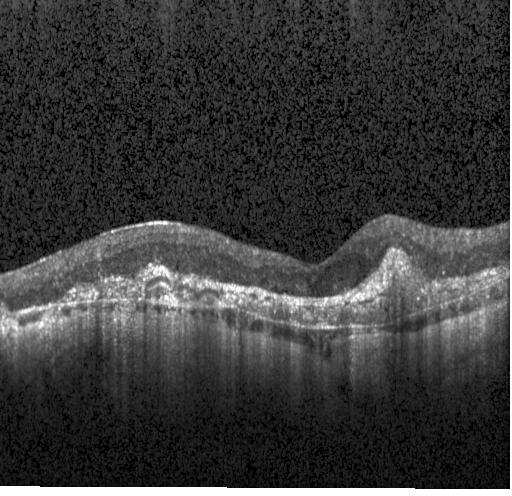 Centered on the fovea, optical coherence tomography scan.
Dx: choroidal neovascularization (CNV).